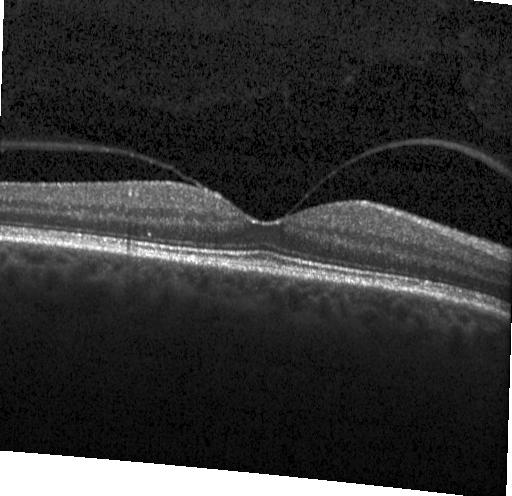 Horizontal scan through the fovea. Optical coherence tomography scan — No choroidal neovascularization, diabetic macular edema, or drusen.